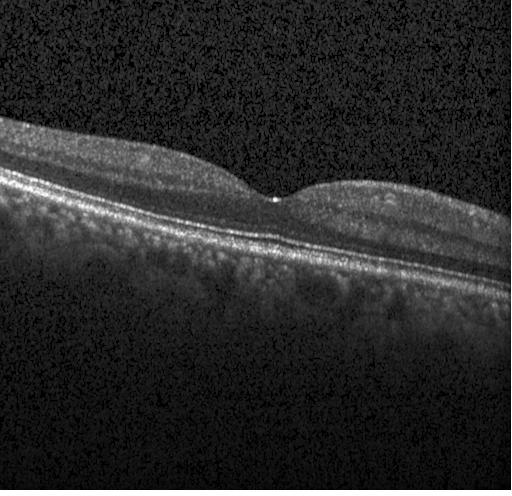
OCT B-scan.
The scan shows neither choroidal neovascularization, diabetic macular edema, nor drusen.